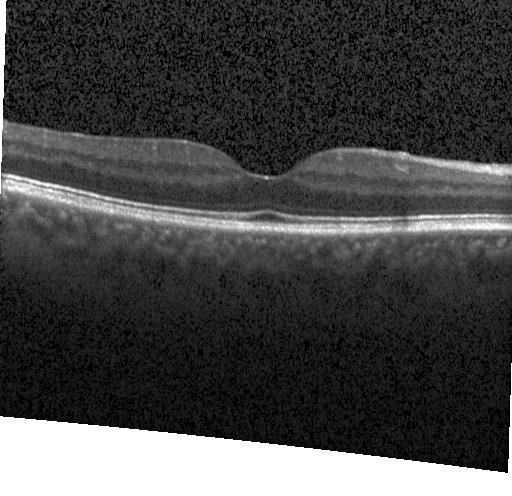

OCT B-scan. Spectral-domain optical coherence tomography. The scan shows no choroidal neovascularization, diabetic macular edema, or drusen.